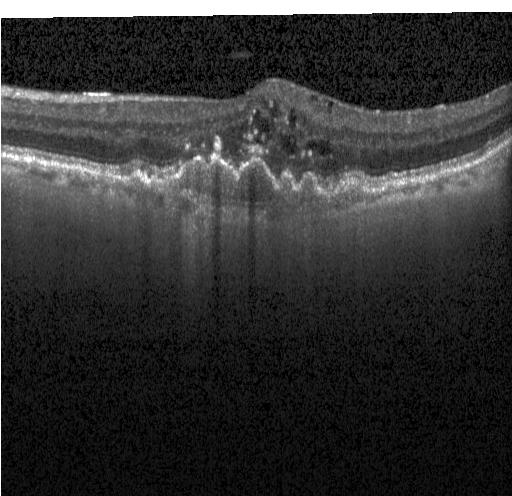

Heidelberg Spectralis OCT system · retinal OCT B-scan · macular scan · spectral-domain OCT — Diagnosis: choroidal neovascularization (CNV).